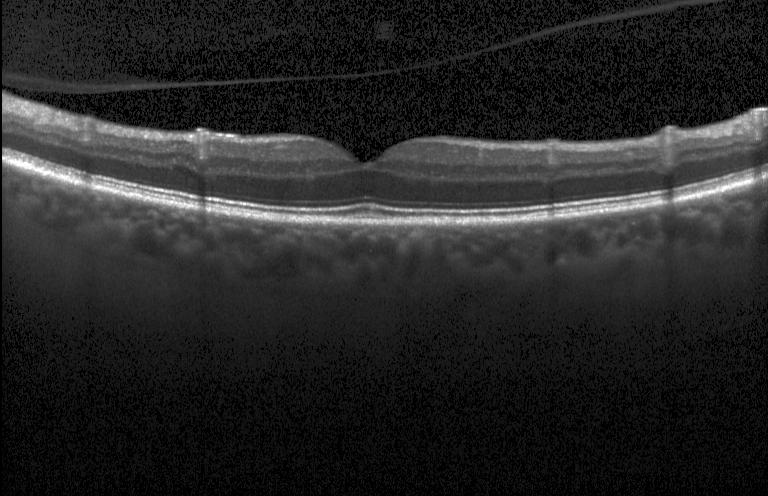
Diagnosis: no evidence of CNV, DME, or drusen.